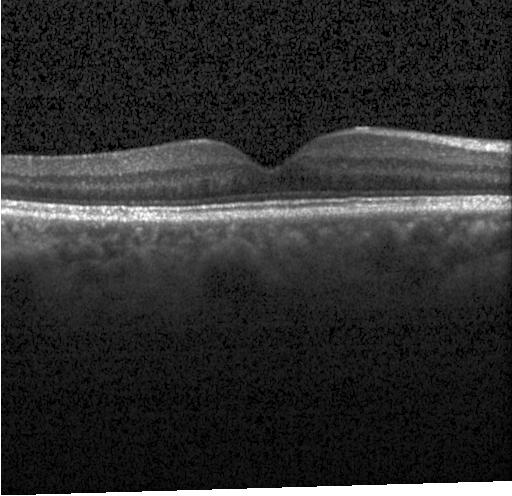
Dx: neither CNV, DME, nor drusen.